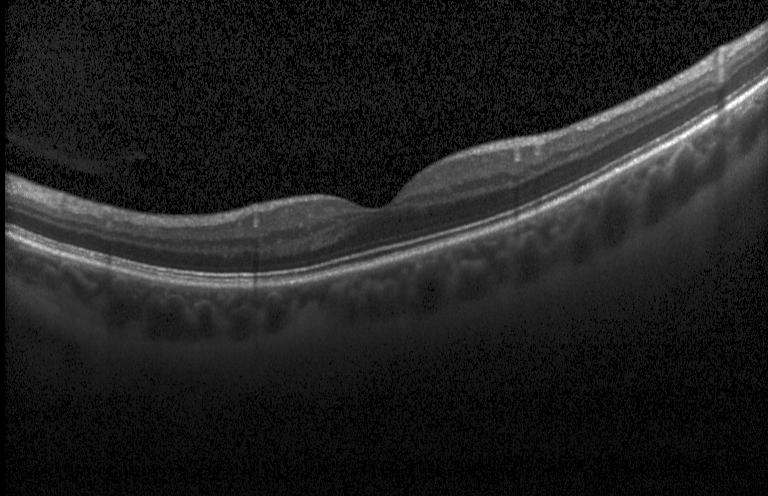 Diagnosis: neither choroidal neovascularization, diabetic macular edema, nor drusen.